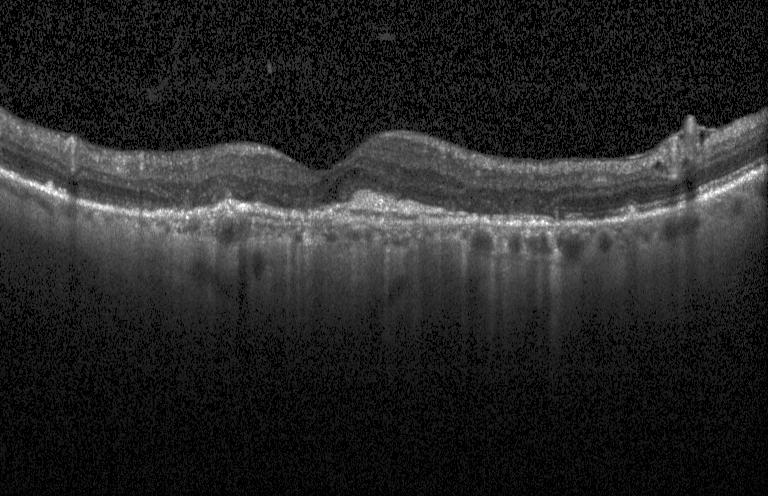
Spectral-domain optical coherence tomography; retinal OCT cross-section
Finding: a choroidal neovascular membrane.